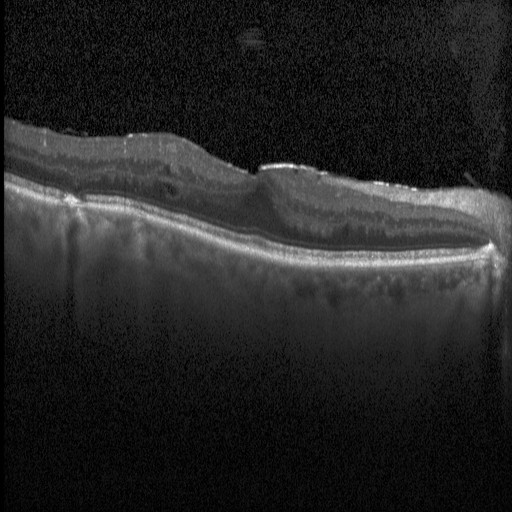
Impression: diabetic macular edema.